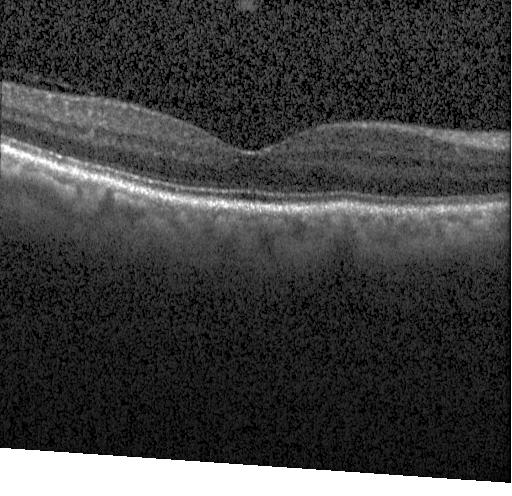 OCT line scan — OCT finding: no choroidal neovascularization, diabetic macular edema, or drusen.